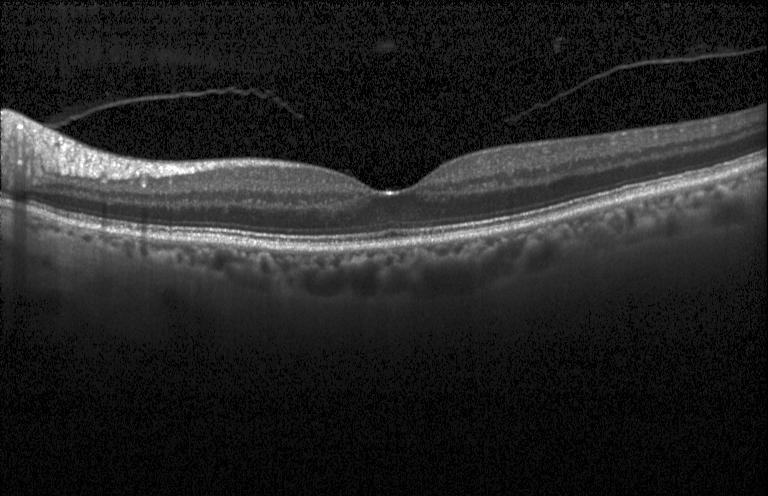
Retinal OCT B-scan · acquired on a Heidelberg Spectralis · SD-OCT — Diagnosis: neither CNV, DME, nor drusen.